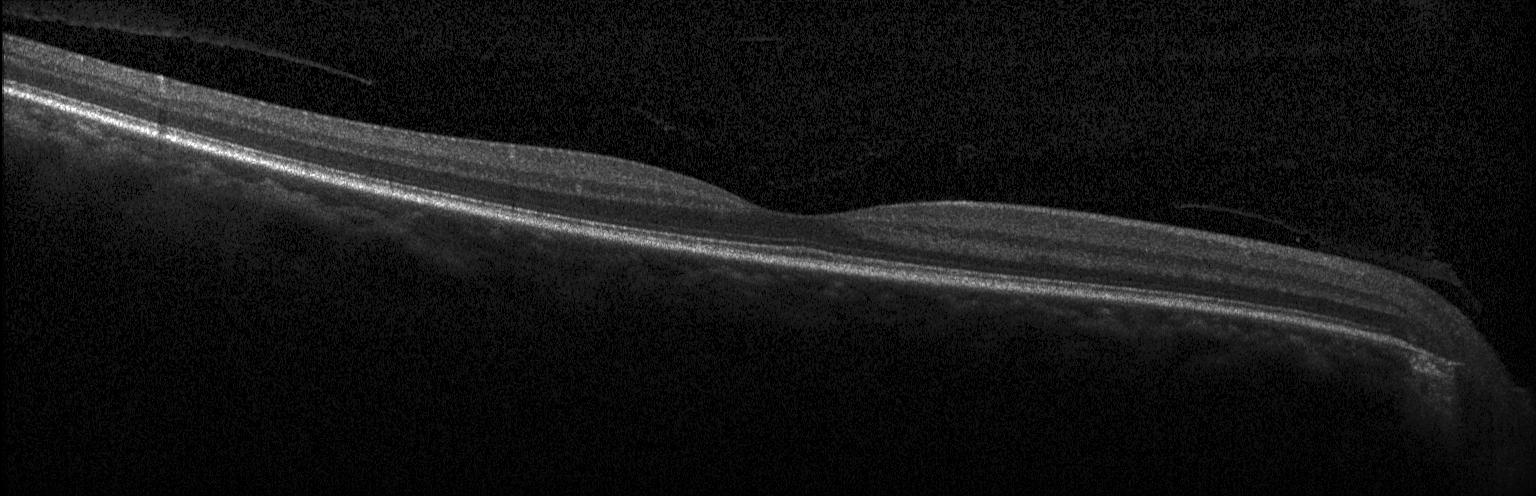

Impression: no CNV, no DME, and no drusen.